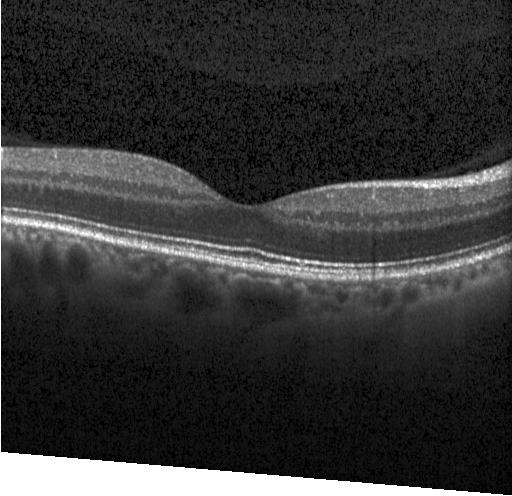
Retinal OCT cross-section, spectral-domain optical coherence tomography
Finding: no evidence of choroidal neovascularization, diabetic macular edema, or drusen.